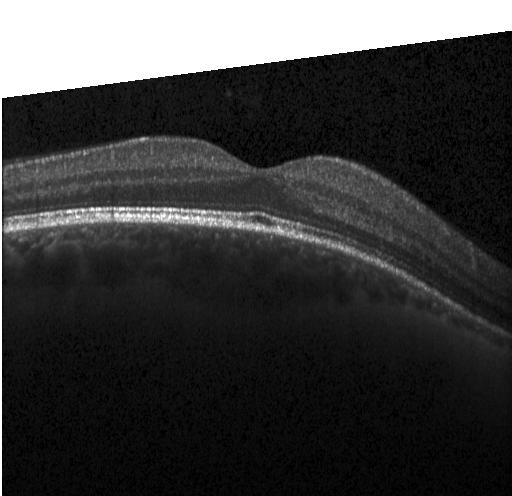

OCT finding: neither choroidal neovascularization, diabetic macular edema, nor drusen.